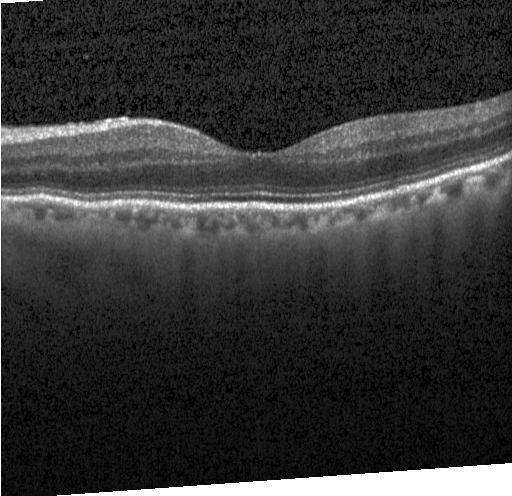 Impression: no choroidal neovascularization, diabetic macular edema, or drusen.